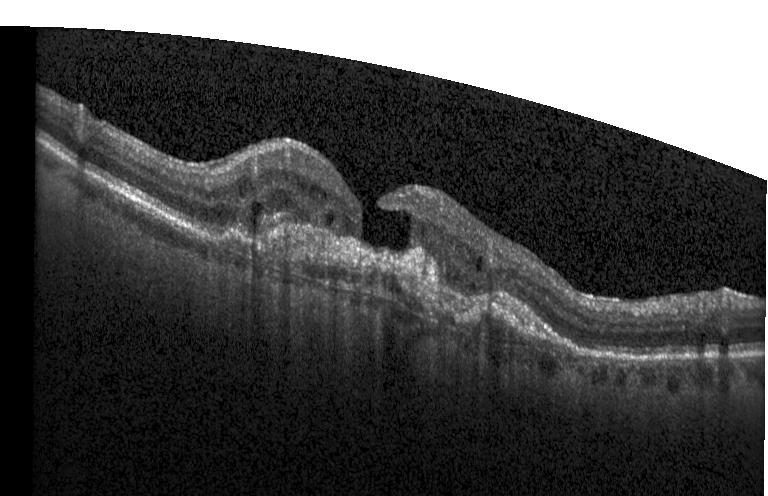 Optical coherence tomography B-scan; instrument: Heidelberg Spectralis; horizontal scan through the fovea. Macular OCT: a choroidal neovascular membrane.